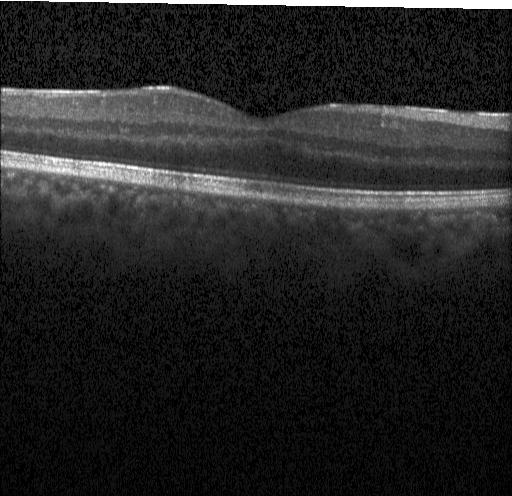
OCT scan showing no choroidal neovascularization, no diabetic macular edema, and no drusen.